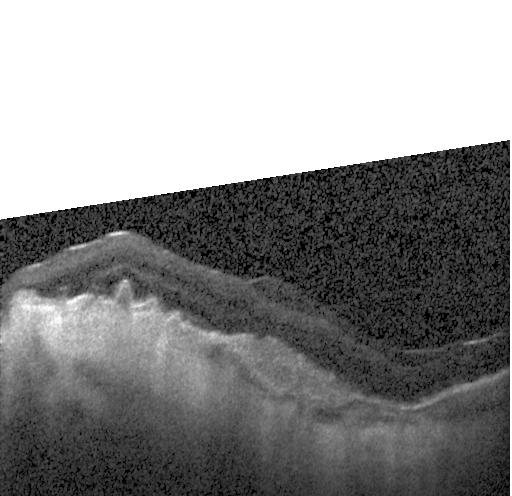 SD-OCT; OCT line scan; horizontal scan through the fovea; acquired on a Heidelberg Spectralis.
A choroidal neovascular membrane.